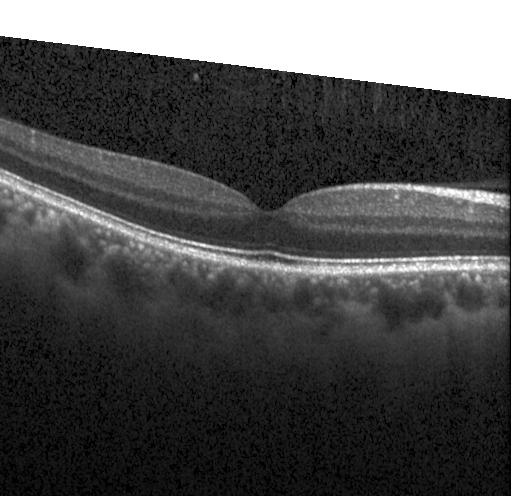
Fovea-centered, OCT B-scan
The scan shows no evidence of choroidal neovascularization, diabetic macular edema, or drusen.